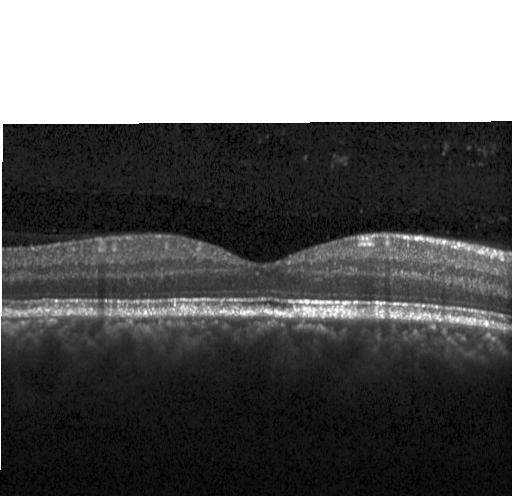
Impression: no choroidal neovascularization, diabetic macular edema, or drusen.